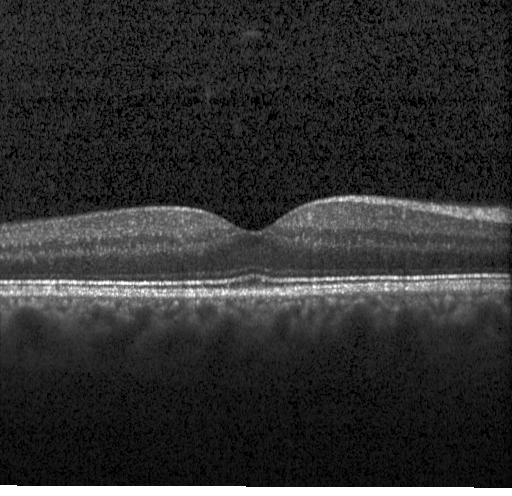 Optical coherence tomography scan
Impression: neither choroidal neovascularization, diabetic macular edema, nor drusen.